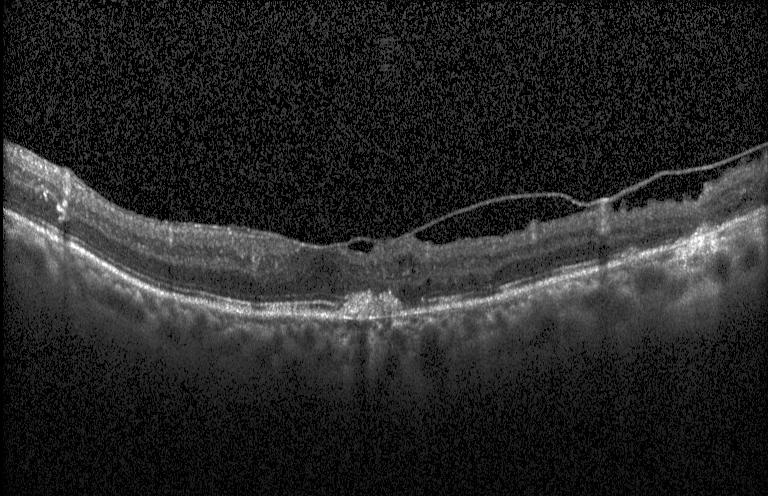
OCT B-scan. SD-OCT. Through the macula. The scan shows a choroidal neovascular membrane.